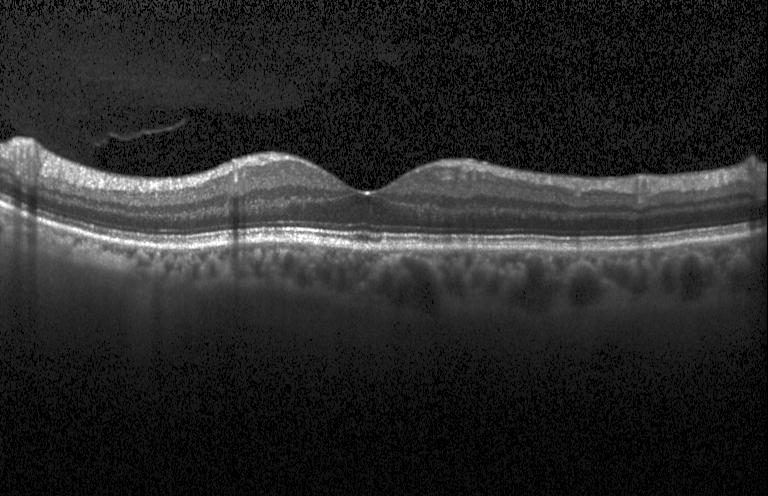 Spectral-domain OCT; centered on the fovea; optical coherence tomography B-scan; acquired on a Heidelberg Spectralis — Assessment: no CNV, no DME, and no drusen.